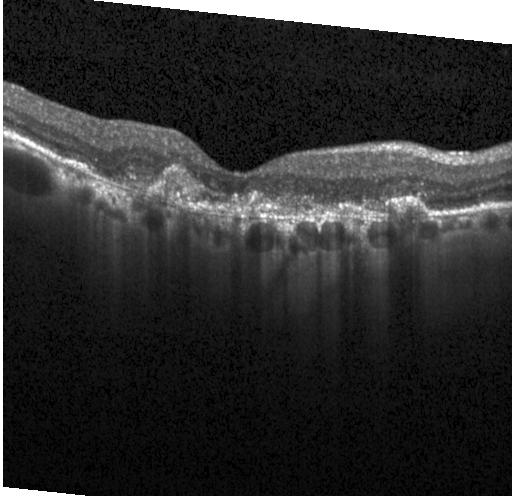
Retinal OCT cross-section · SD-OCT.
Macular OCT: CNV.